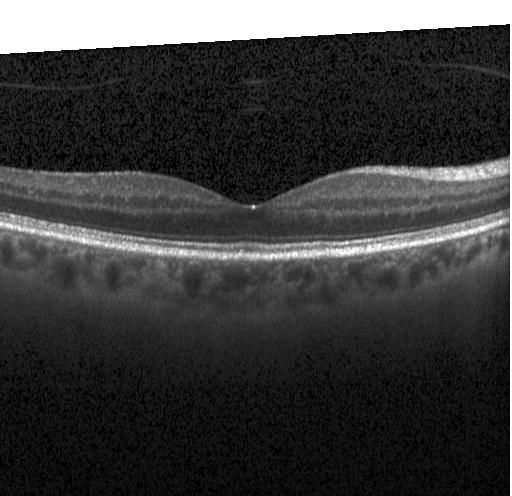

OCT scan showing no choroidal neovascularization, no diabetic macular edema, and no drusen.